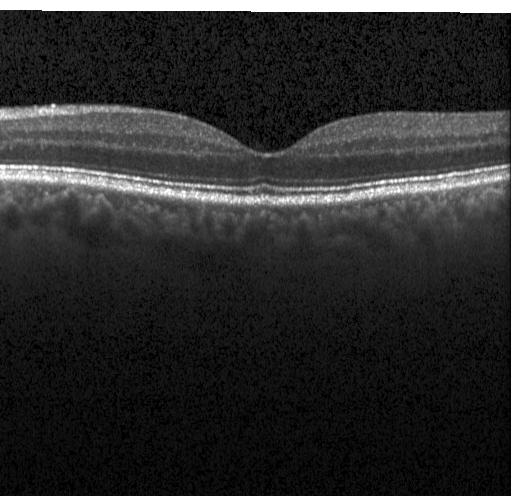

Assessment: neither choroidal neovascularization, diabetic macular edema, nor drusen.